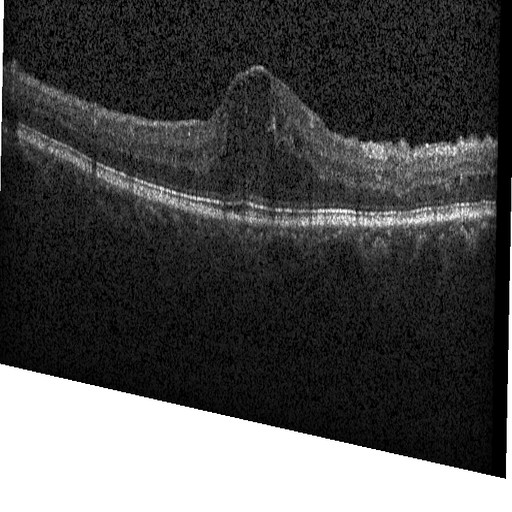 Dx: DME.